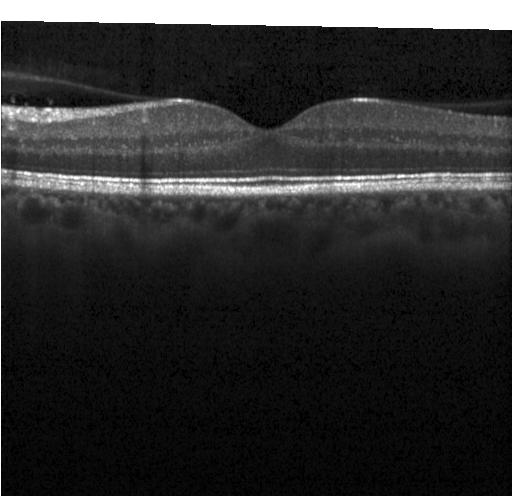 Spectral-domain optical coherence tomography · Heidelberg Spectralis · optical coherence tomography scan · centered on the fovea. Assessment: neither CNV, DME, nor drusen.